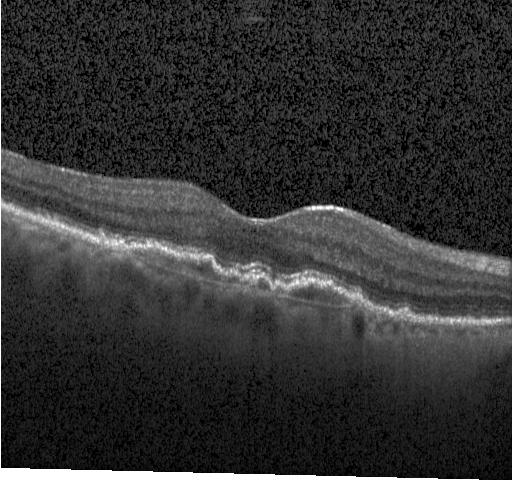
Dx: a choroidal neovascular membrane.